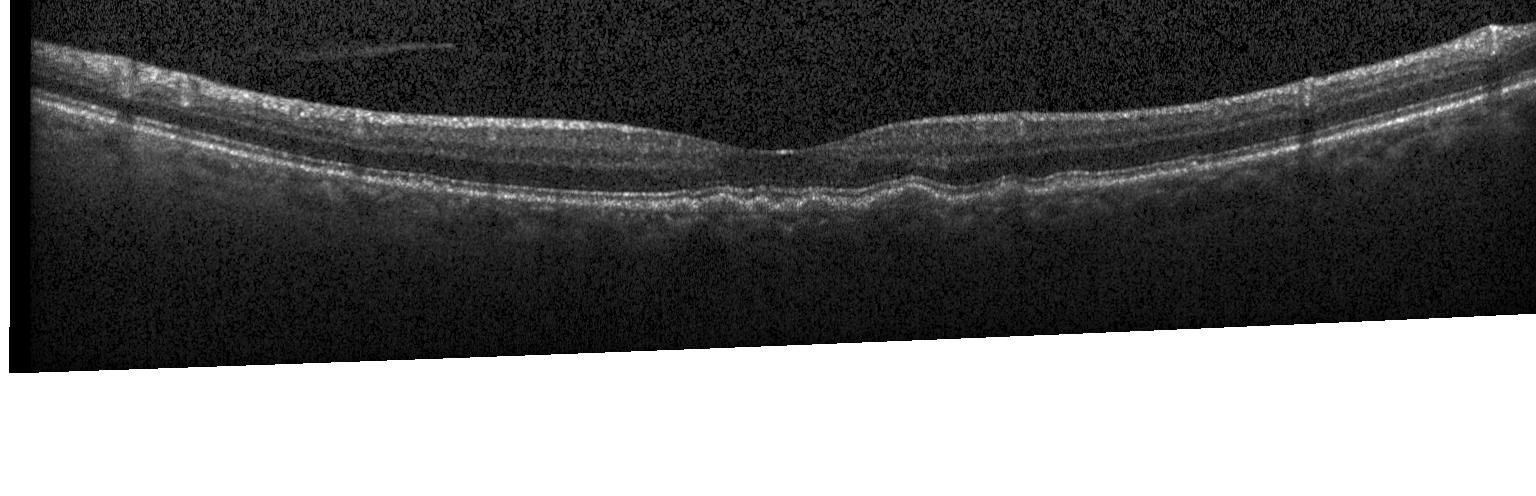

Spectral-domain OCT. Horizontal scan through the fovea. Acquired on a Heidelberg Spectralis. Optical coherence tomography scan — Assessment: sub-RPE drusenoid deposits.